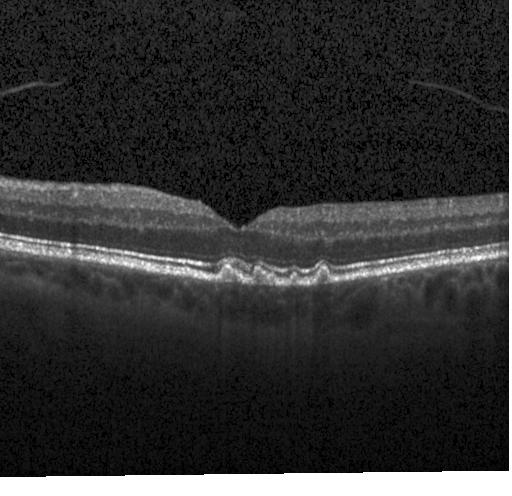 Dx: sub-RPE drusenoid deposits.